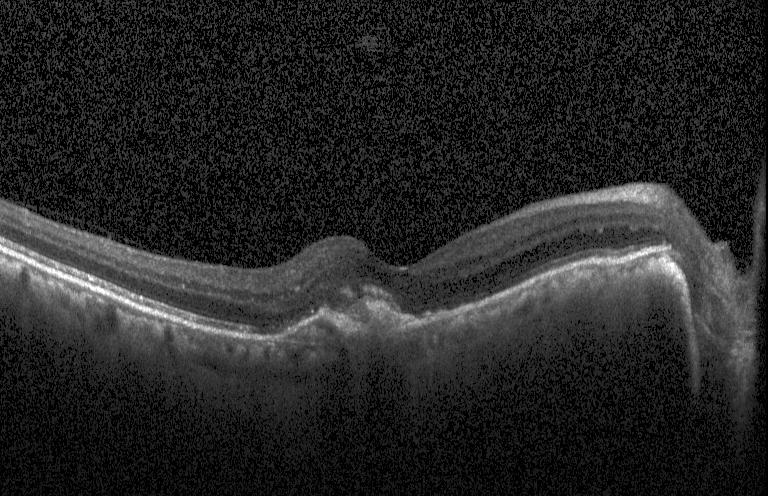 OCT line scan. Macular scan. SD-OCT. Impression: choroidal neovascularization (CNV).